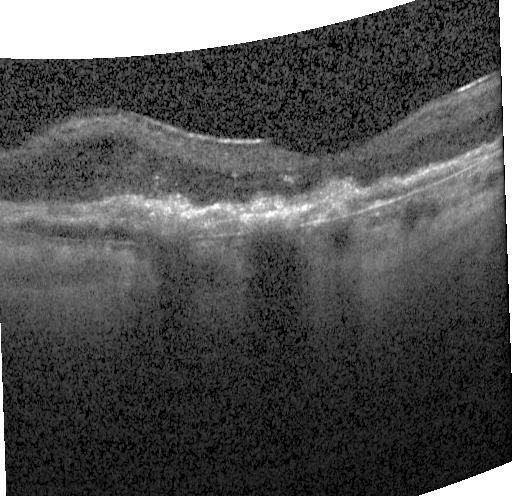

Spectral-domain OCT; OCT line scan; Heidelberg Spectralis OCT system.
The scan shows a choroidal neovascular membrane.